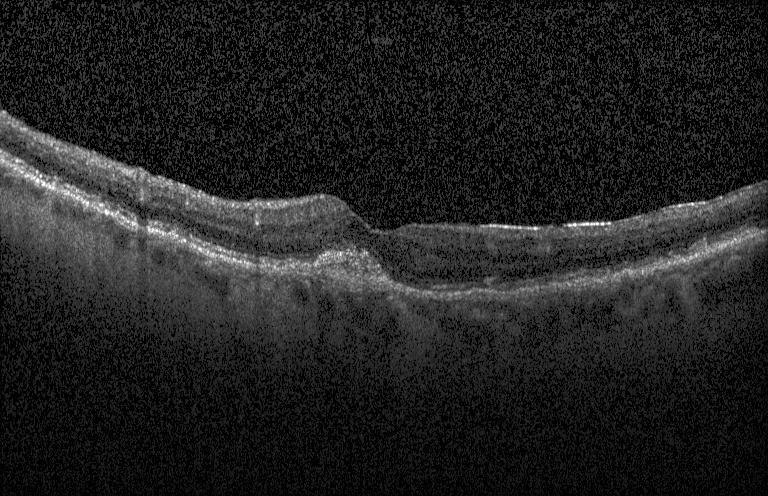

OCT line scan · acquired on a Heidelberg Spectralis.
Finding: a choroidal neovascular membrane.